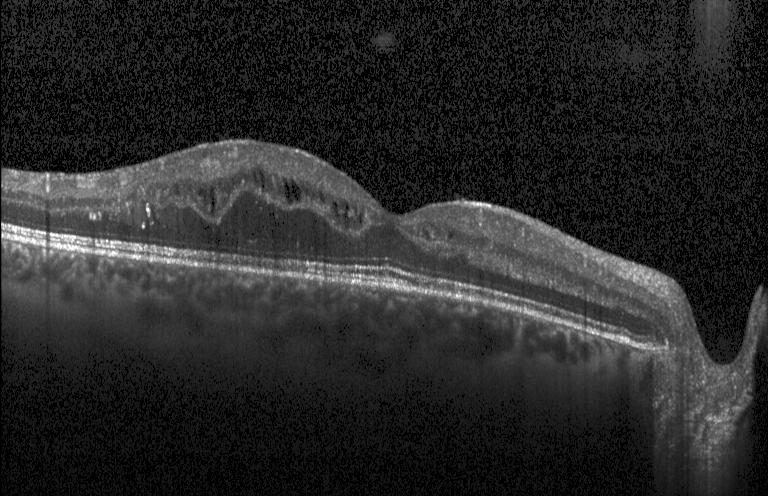 Spectral-domain optical coherence tomography. Heidelberg Spectralis. Retinal OCT B-scan — This B-scan demonstrates diabetic macular edema (DME).